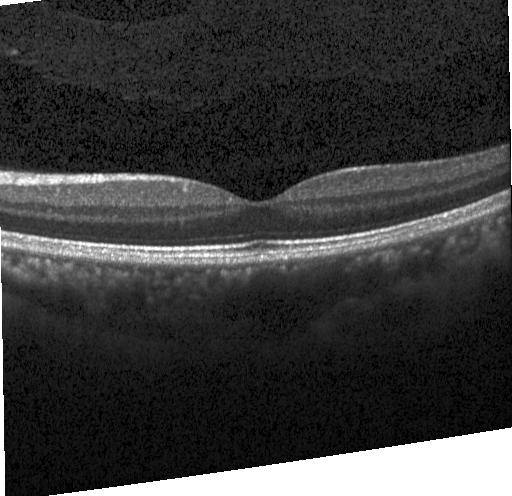
Centered on the fovea, optical coherence tomography scan, acquired on a Heidelberg Spectralis. Macular OCT: no choroidal neovascularization, diabetic macular edema, or drusen.